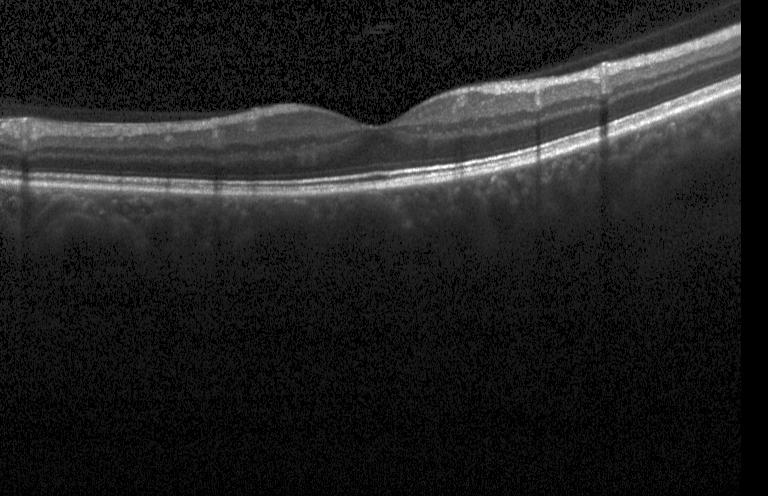

OCT B-scan; Heidelberg Spectralis. Diagnosis: neither choroidal neovascularization, diabetic macular edema, nor drusen.